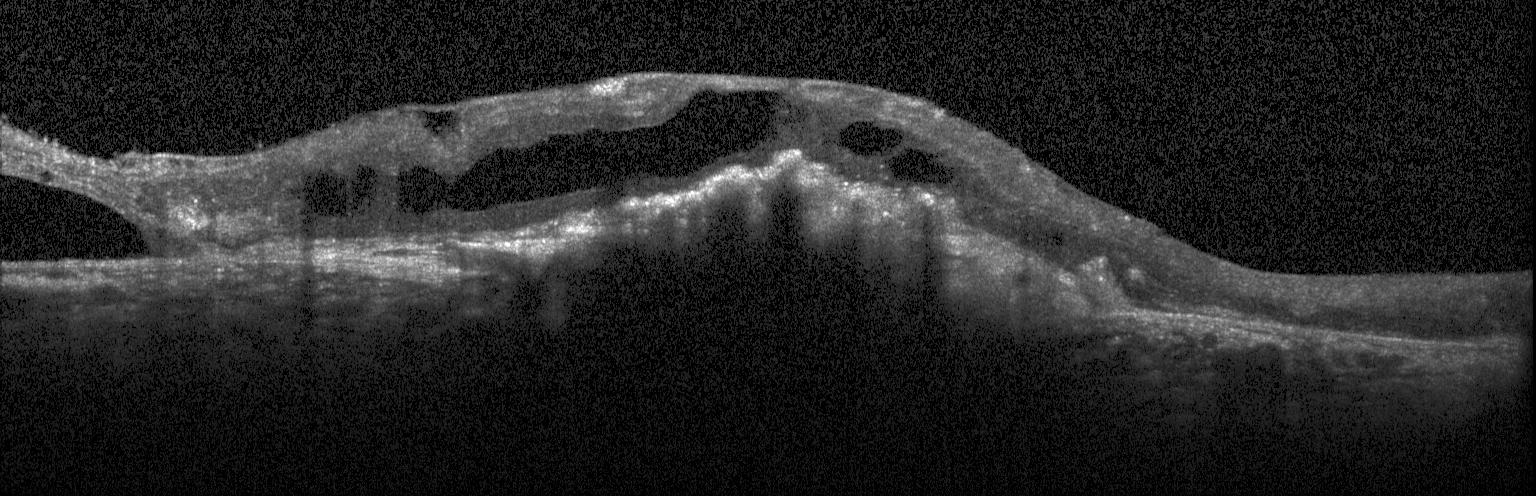 Finding: a choroidal neovascular membrane.